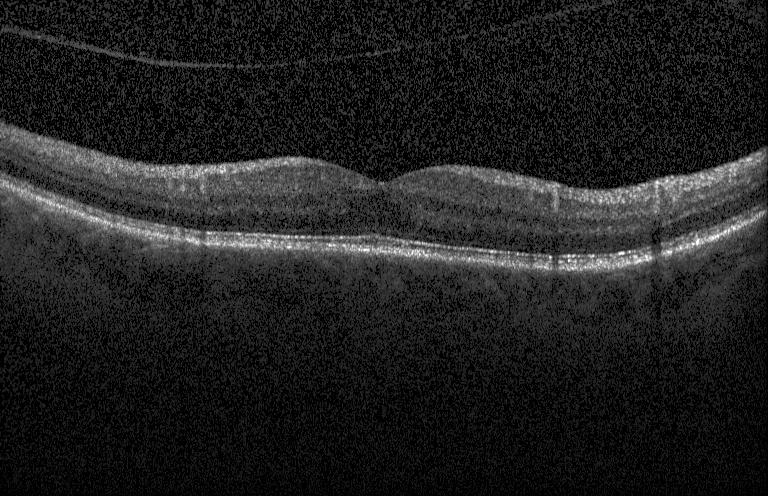 Optical coherence tomography scan, acquired on a Heidelberg Spectralis, horizontal scan through the fovea, spectral-domain optical coherence tomography. No choroidal neovascularization, diabetic macular edema, or drusen.